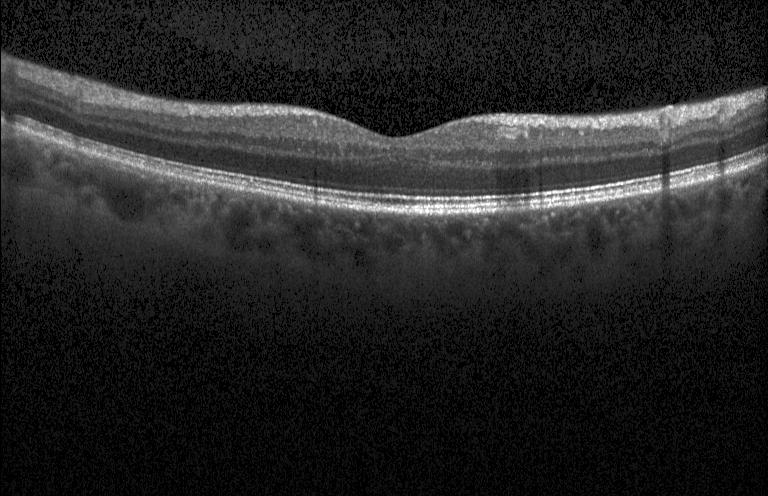 Retinal OCT cross-section showing no CNV, no DME, and no drusen.